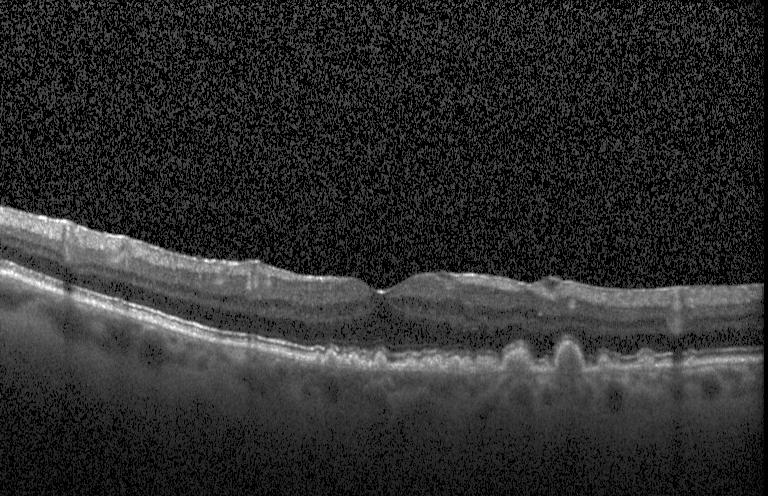

Assessment: sub-RPE drusenoid deposits.